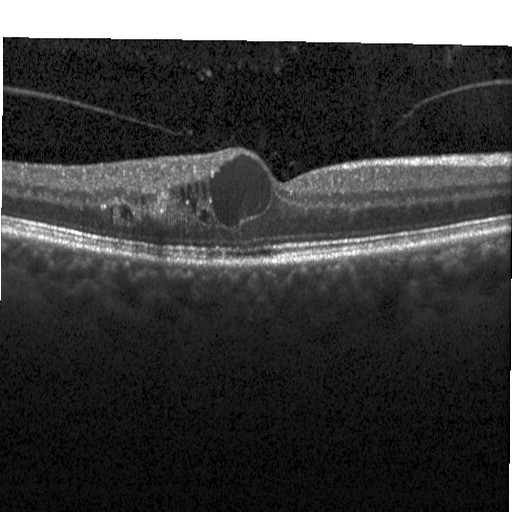
Impression: diabetic macular edema.